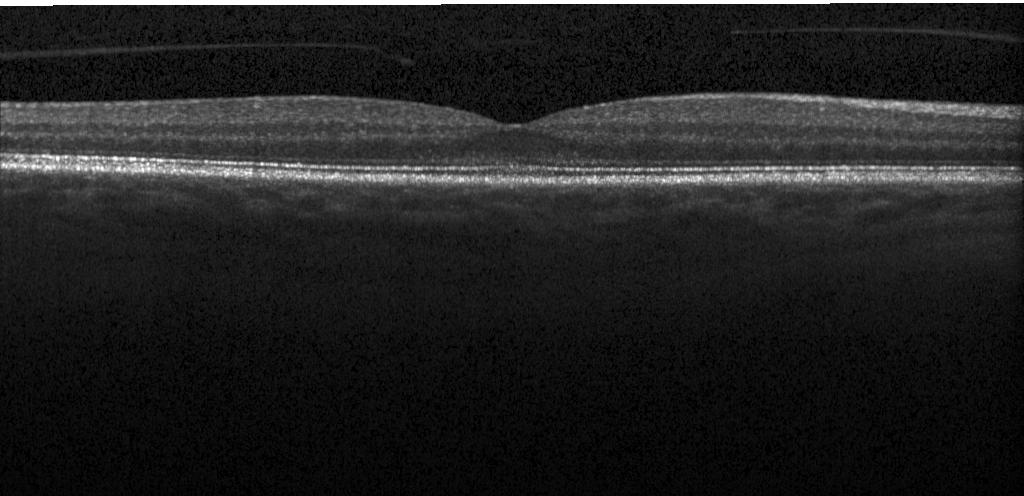 Diagnosis: no choroidal neovascularization, no diabetic macular edema, and no drusen.